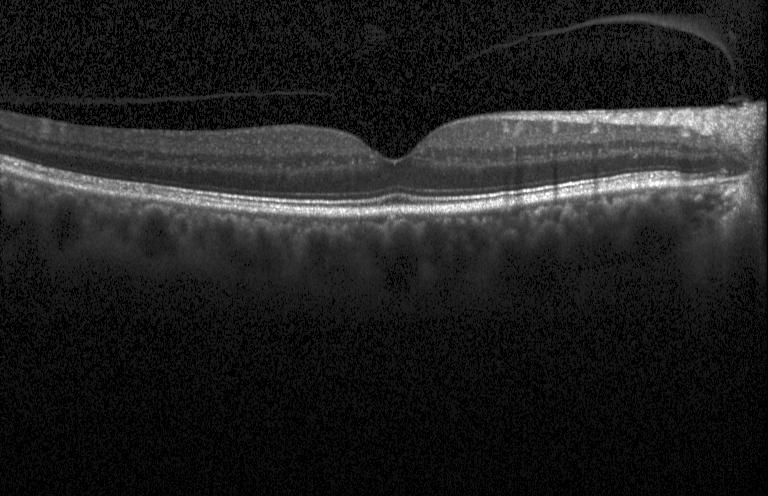 OCT B-scan. This B-scan demonstrates no evidence of choroidal neovascularization, diabetic macular edema, or drusen.